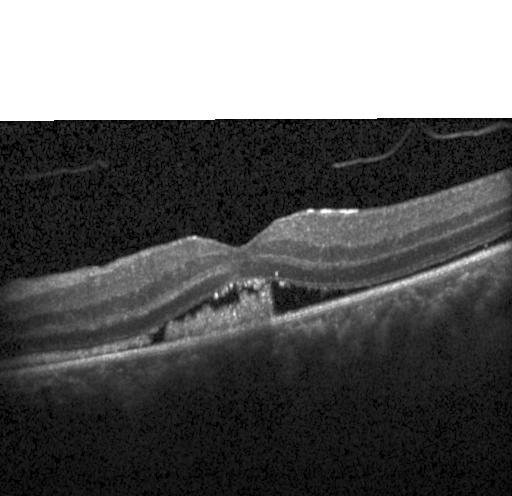 Optical coherence tomography B-scan
Finding: a choroidal neovascular membrane.